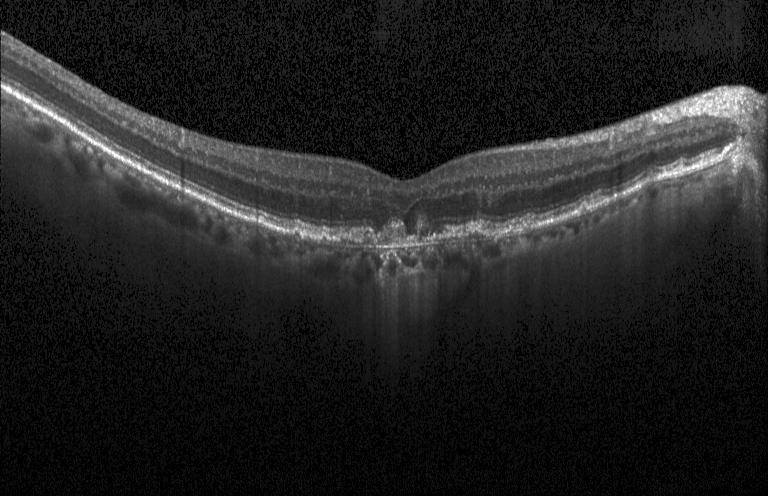 Retinal OCT cross-section.
Impression: CNV.